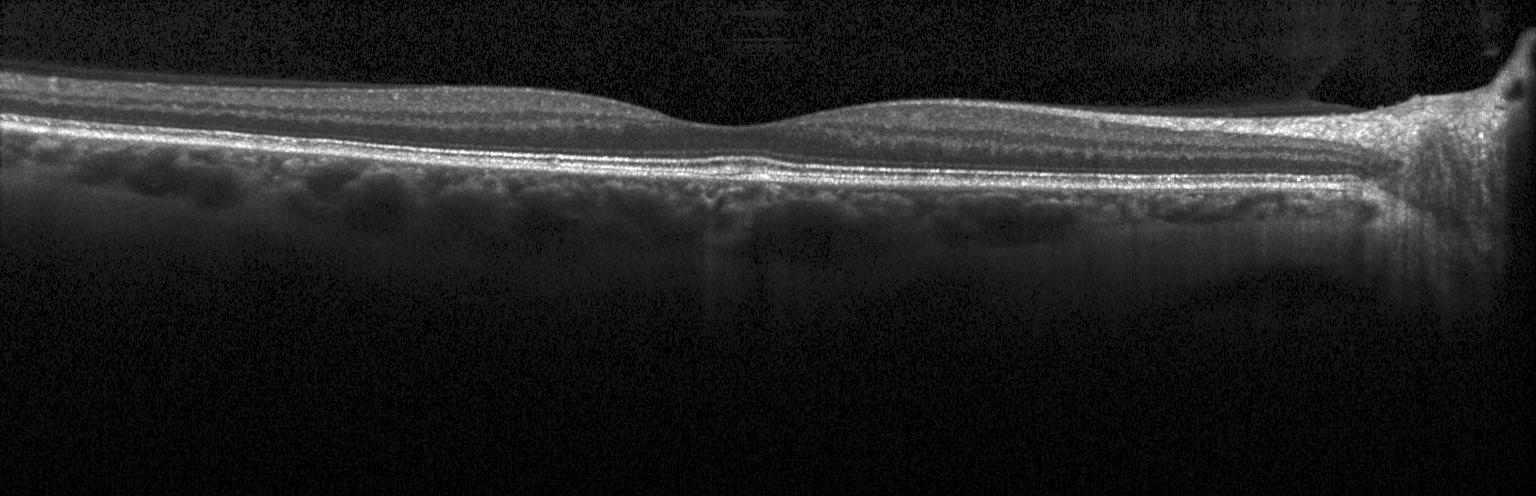 Finding: neither choroidal neovascularization, diabetic macular edema, nor drusen.